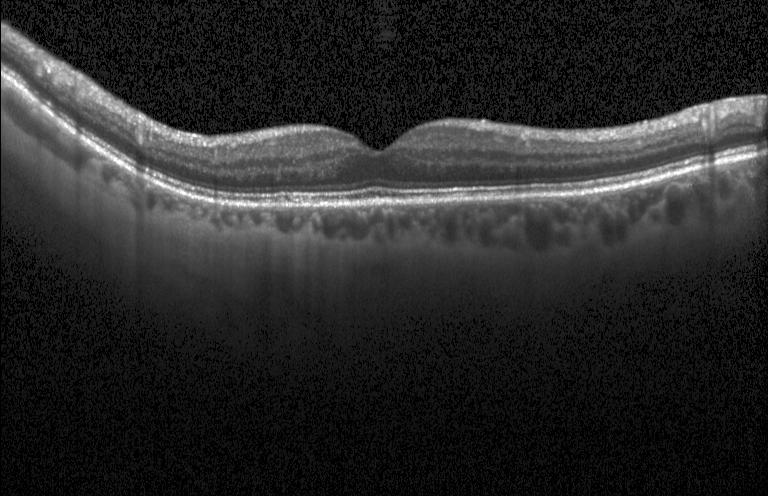

Heidelberg Spectralis, spectral-domain optical coherence tomography, optical coherence tomography B-scan, horizontal scan through the fovea.
Finding: no choroidal neovascularization, no diabetic macular edema, and no drusen.